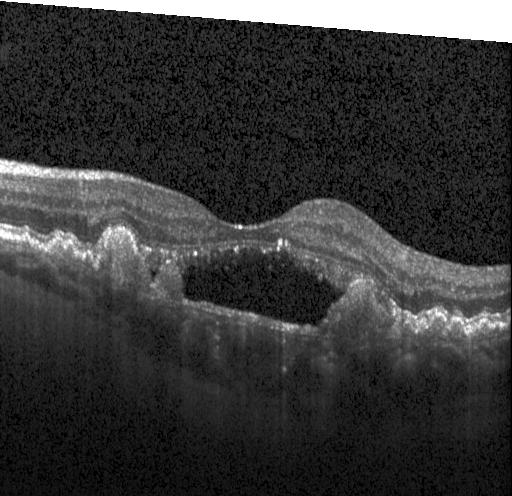

Heidelberg Spectralis OCT system · fovea-centered · retinal OCT B-scan · SD-OCT. Assessment: a choroidal neovascular membrane.